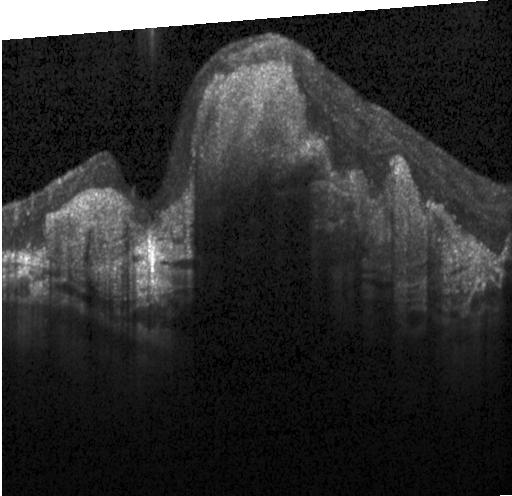 OCT line scan. Spectral-domain optical coherence tomography — Finding: a choroidal neovascular membrane.